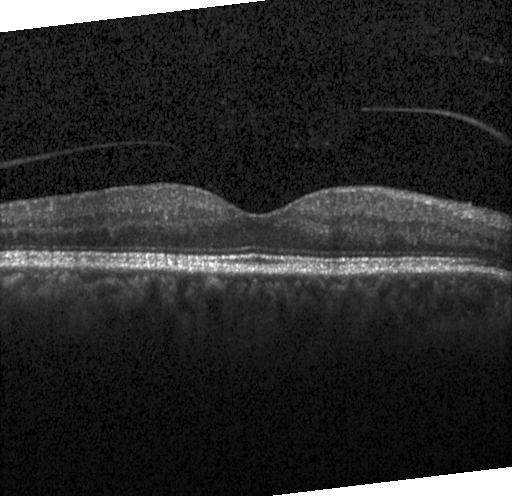 Macular OCT: no evidence of CNV, DME, or drusen.